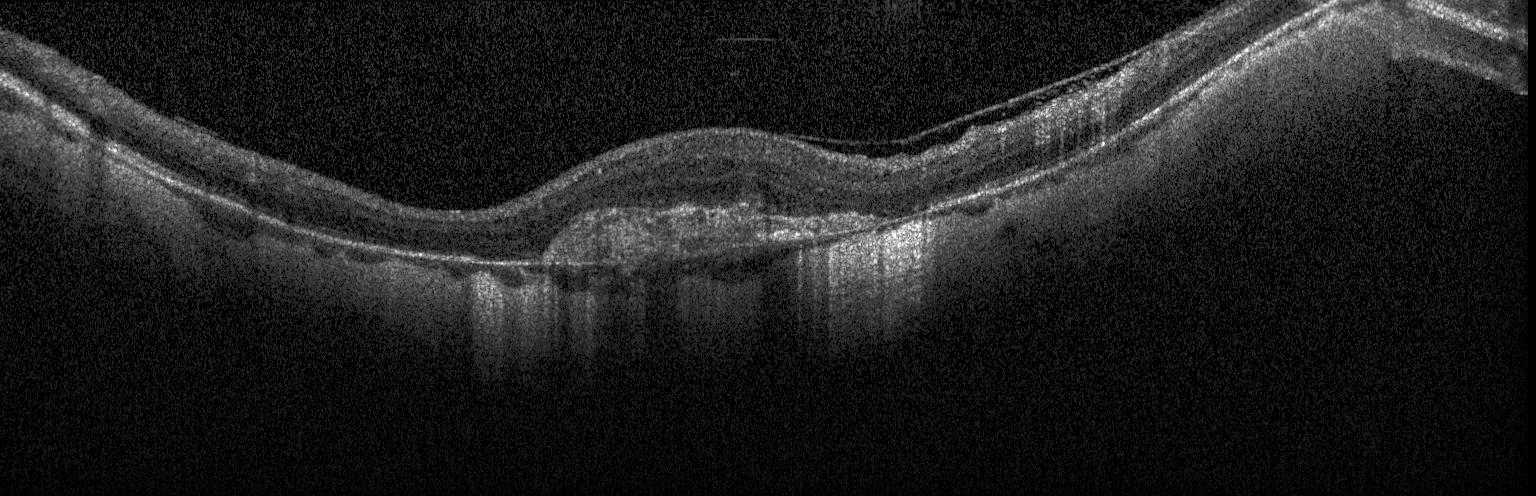 Retinal OCT B-scan.
The scan shows CNV.